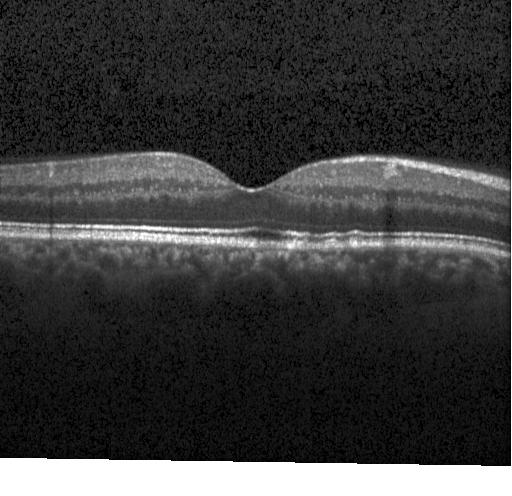

SD-OCT; retinal OCT B-scan
Impression: drusen.